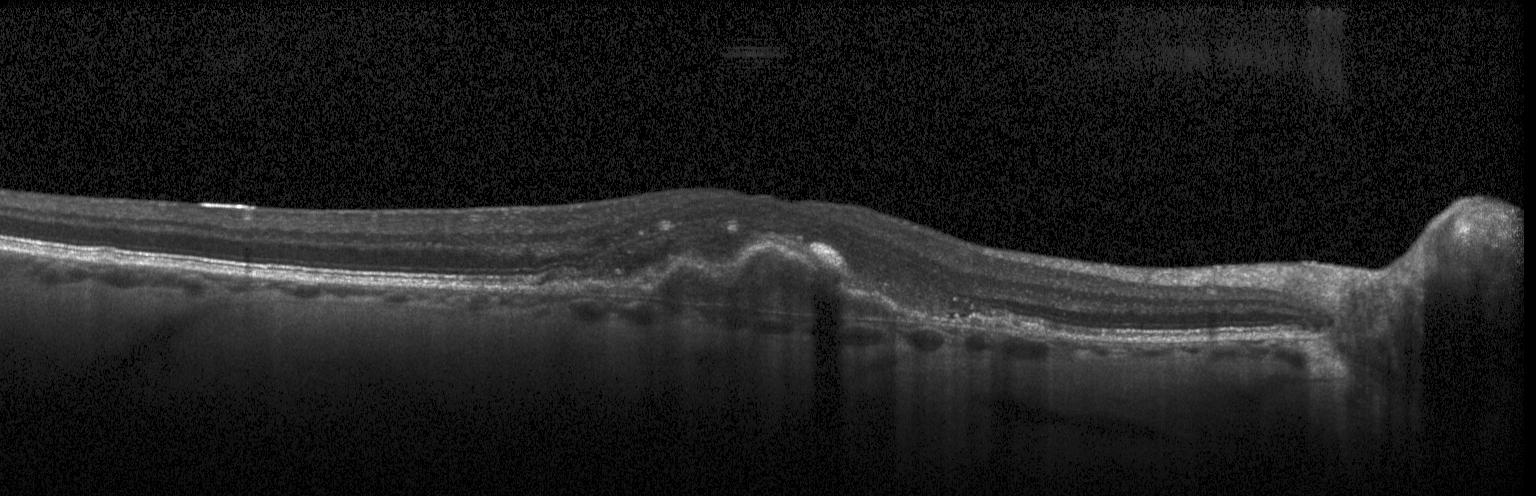

Centered on the fovea, instrument: Heidelberg Spectralis, spectral-domain optical coherence tomography, optical coherence tomography scan — Finding: choroidal neovascularization (CNV).